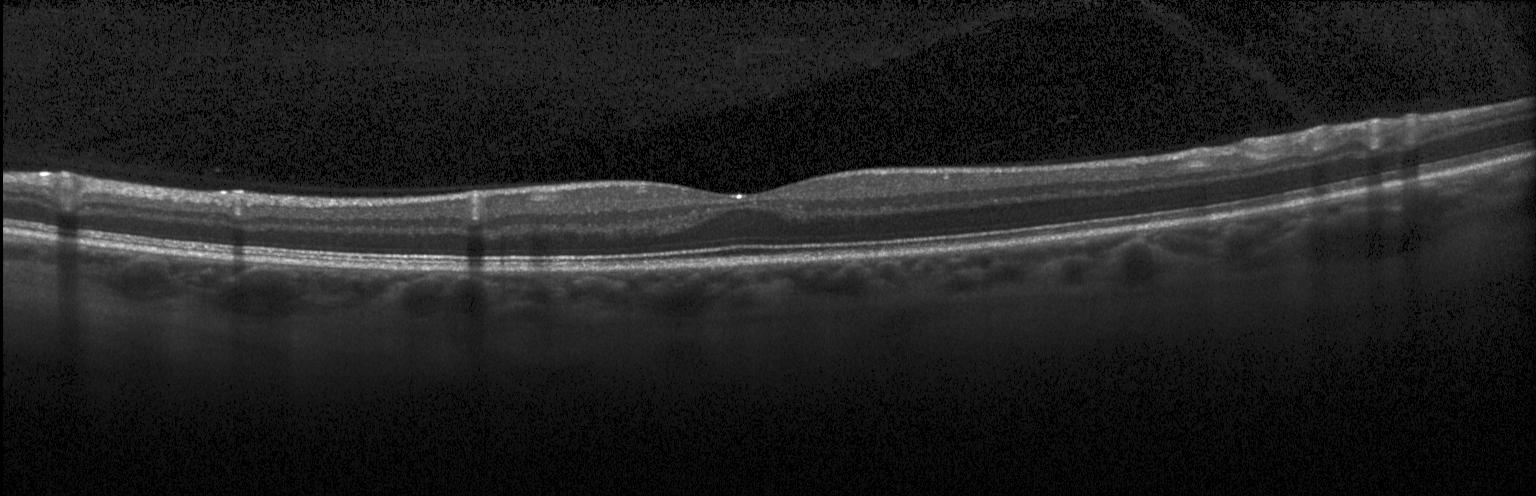

Spectral-domain OCT B-scan: no choroidal neovascularization, diabetic macular edema, or drusen.